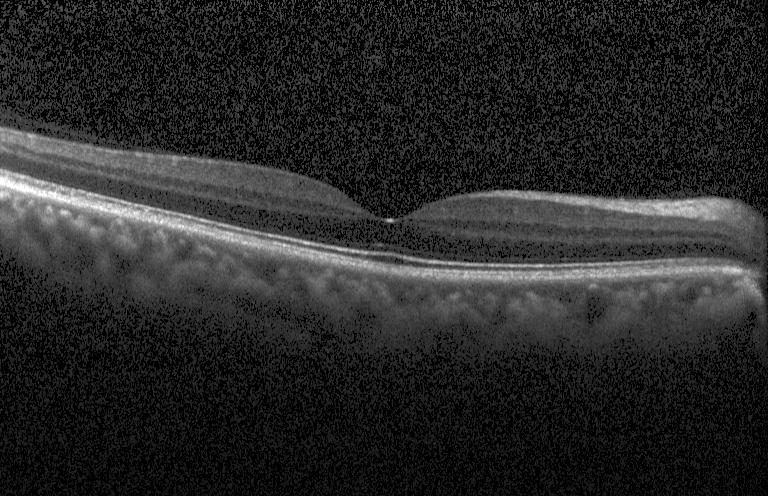 The scan shows no evidence of choroidal neovascularization, diabetic macular edema, or drusen.